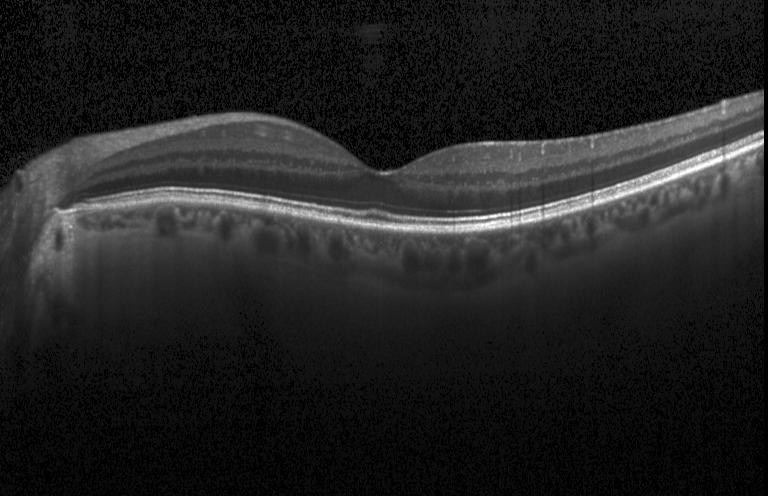
Heidelberg Spectralis OCT system. Spectral-domain optical coherence tomography. OCT B-scan. Macular scan.
Finding: no choroidal neovascularization, diabetic macular edema, or drusen.